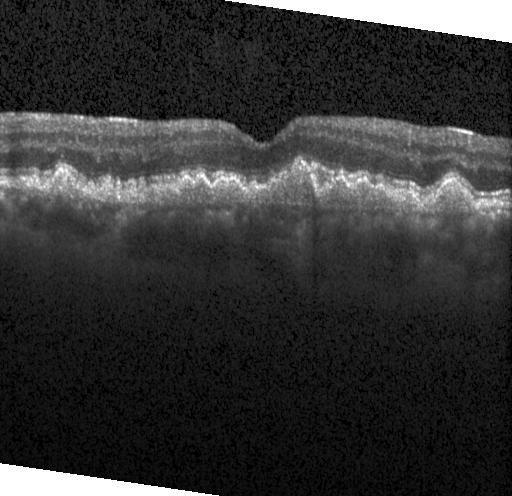 Optical coherence tomography B-scan, spectral-domain optical coherence tomography, through the macula, instrument: Heidelberg Spectralis. Assessment: CNV.